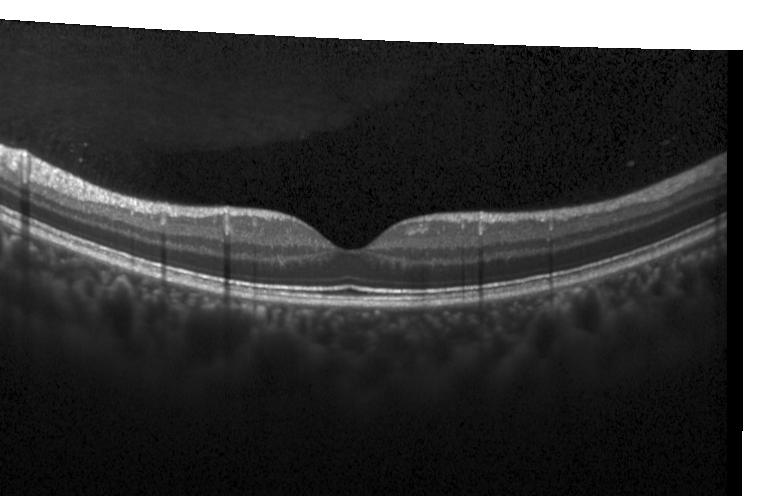

OCT B-scan; instrument: Heidelberg Spectralis; spectral-domain OCT
Assessment: no evidence of CNV, DME, or drusen.